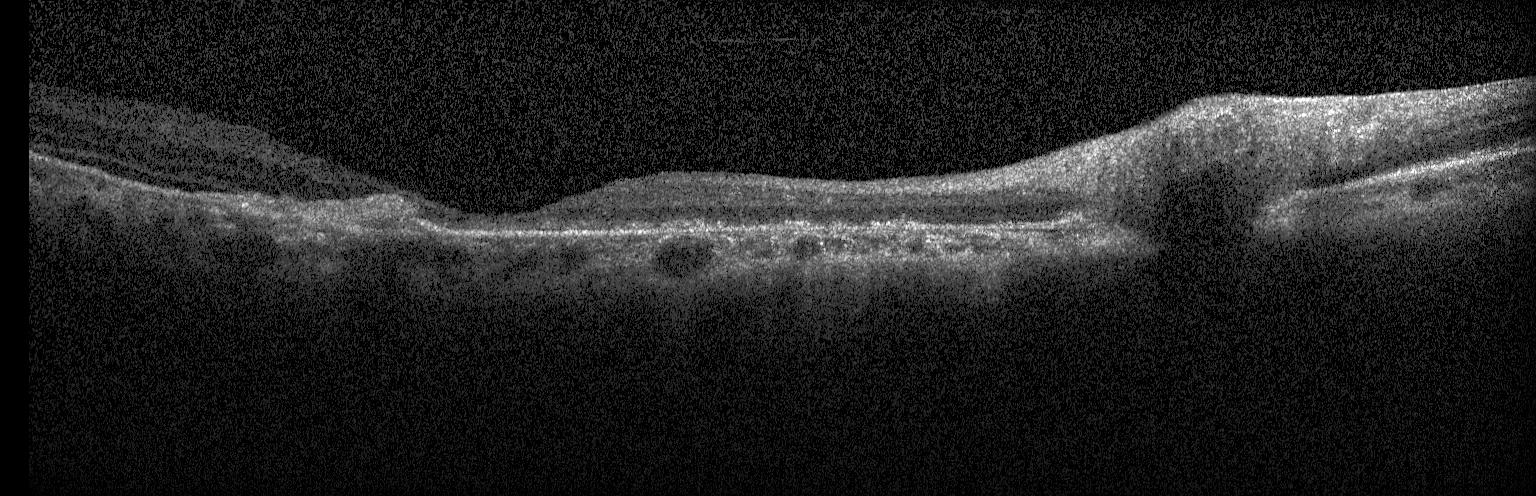 Dx: choroidal neovascularization.